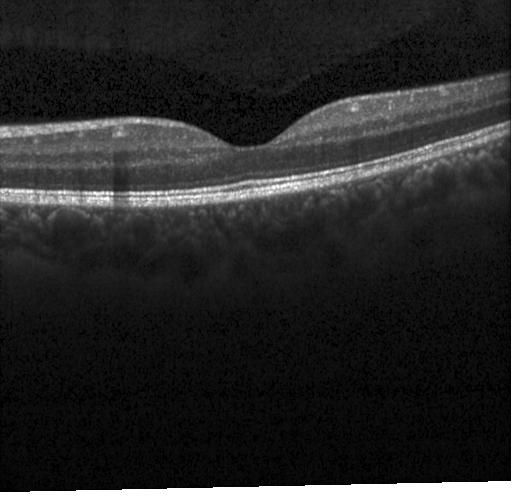
The scan shows no choroidal neovascularization, no diabetic macular edema, and no drusen.